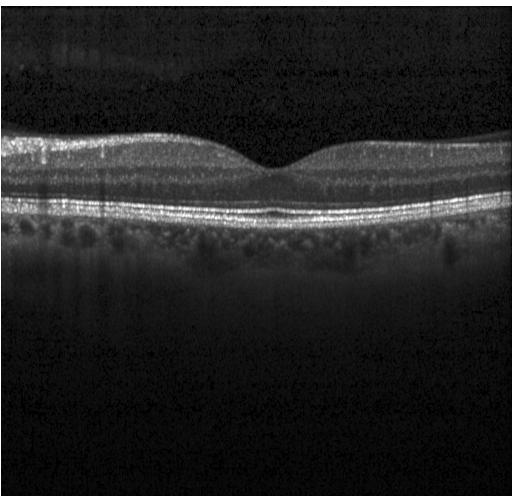
No CNV, DME, or drusen.